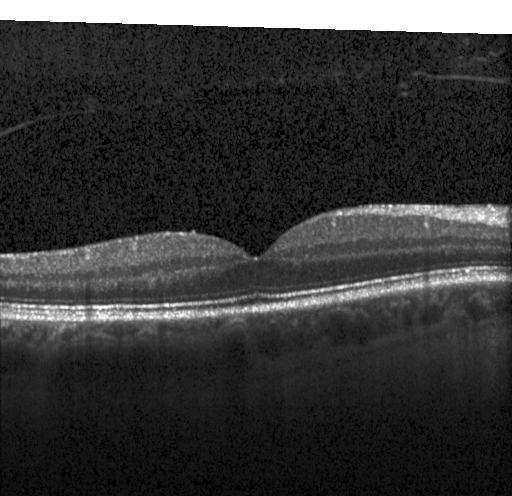
Horizontal scan through the fovea; optical coherence tomography B-scan; SD-OCT; instrument: Heidelberg Spectralis — Assessment: no evidence of CNV, DME, or drusen.